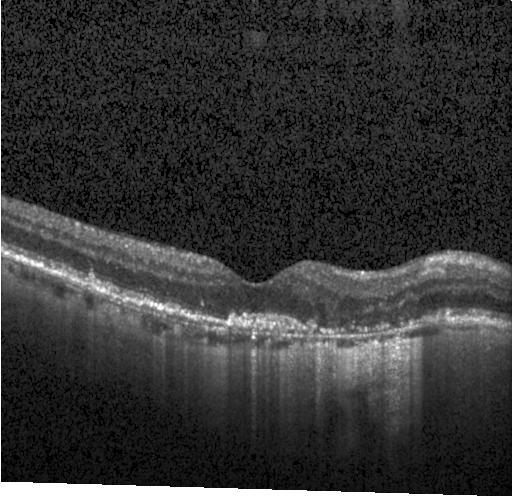
Diagnosis: a choroidal neovascular membrane.